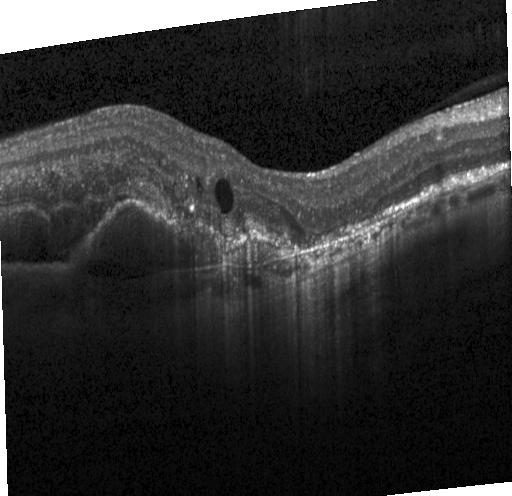
Retinal OCT cross-section — Impression: a choroidal neovascular membrane.